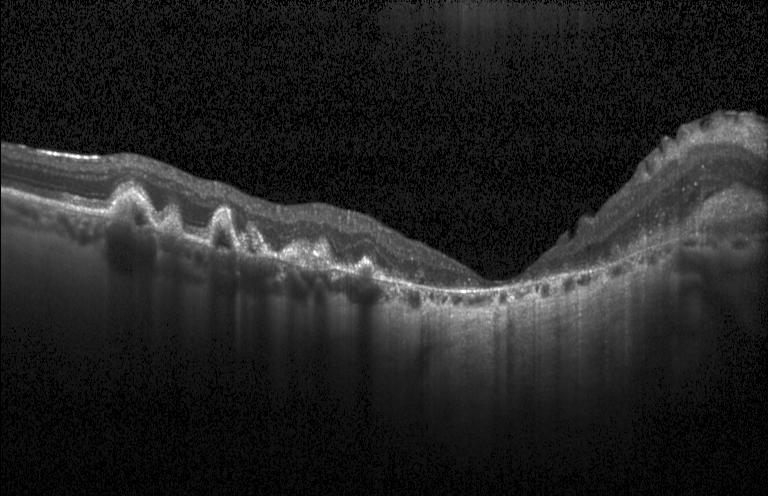

Optical coherence tomography scan, SD-OCT
Assessment: a choroidal neovascular membrane.